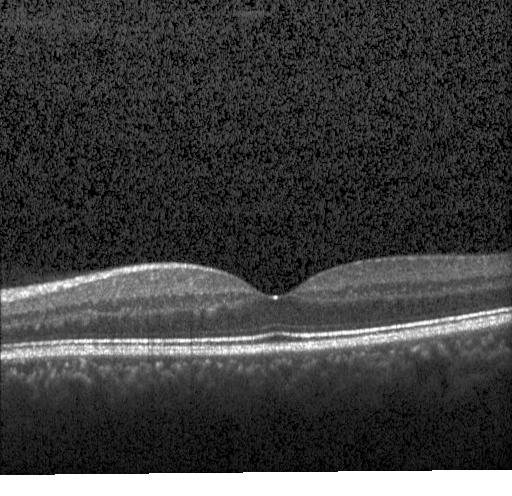 Retinal OCT B-scan, acquired on a Heidelberg Spectralis.
Diagnosis: no evidence of choroidal neovascularization, diabetic macular edema, or drusen.